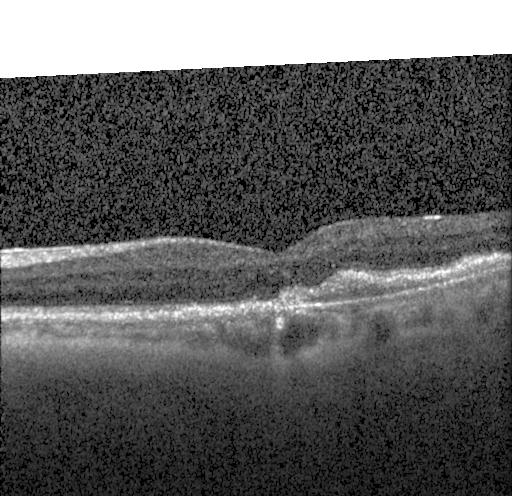

This B-scan demonstrates a choroidal neovascular membrane.